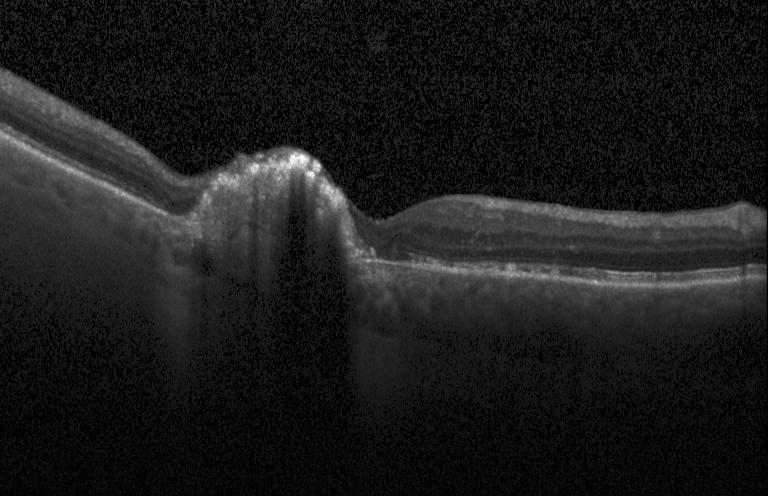 OCT line scan; horizontal scan through the fovea; SD-OCT; acquired on a Heidelberg Spectralis.
Finding: CNV.